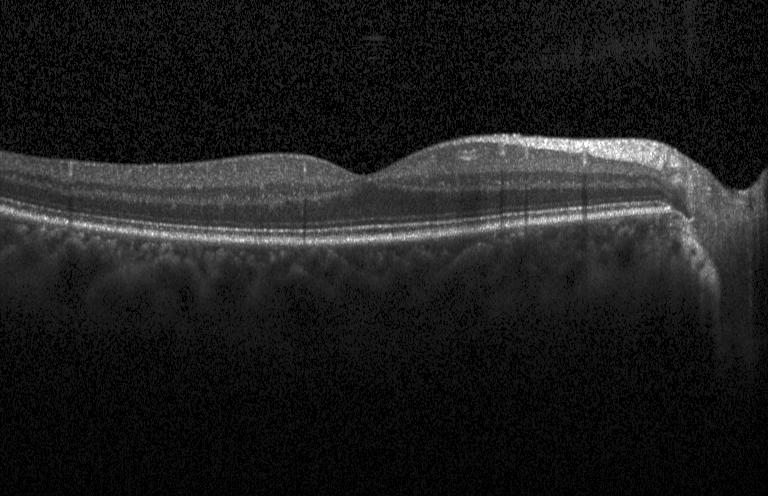

Spectral-domain OCT; retinal OCT cross-section — Impression: no evidence of choroidal neovascularization, diabetic macular edema, or drusen.